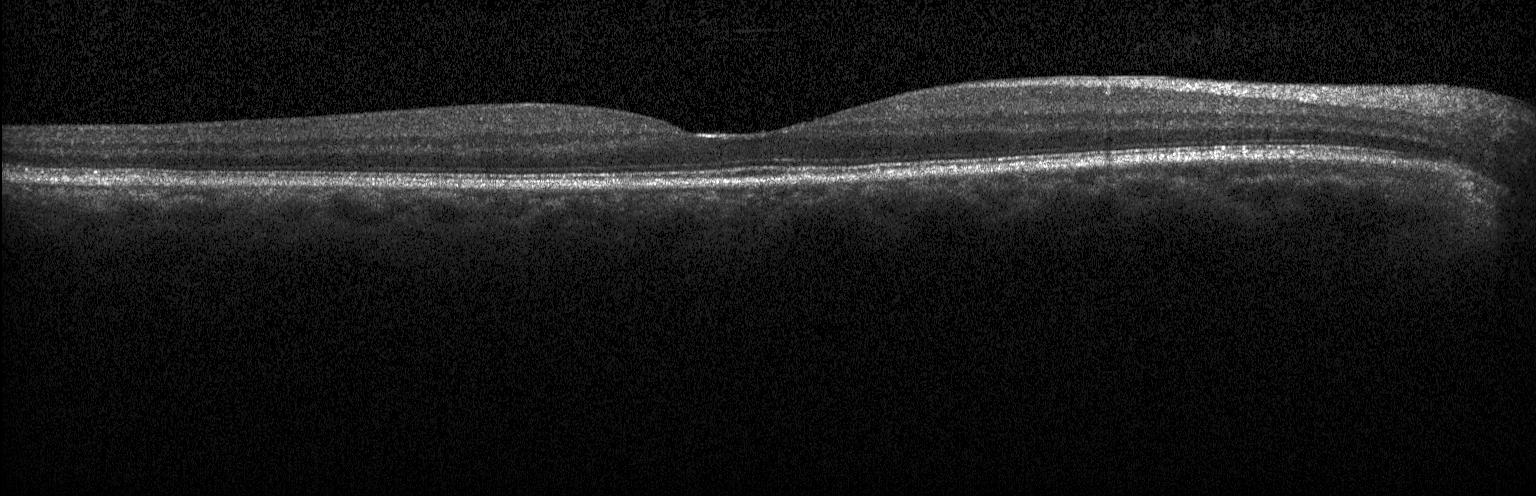 Macular scan; SD-OCT; retinal OCT B-scan
OCT finding: no evidence of choroidal neovascularization, diabetic macular edema, or drusen.